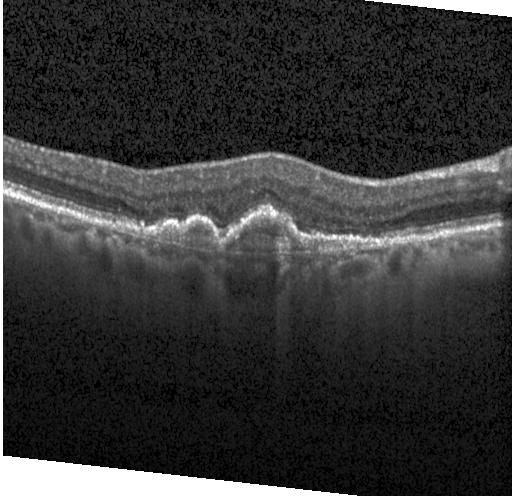
Assessment: a choroidal neovascular membrane.